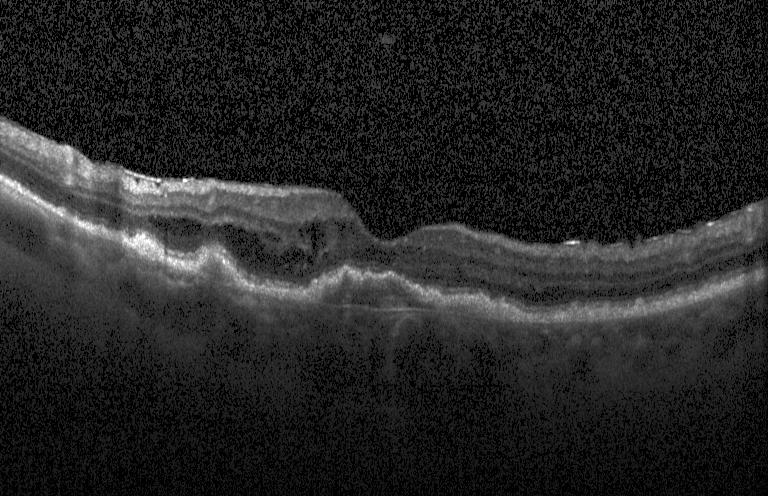
Optical coherence tomography scan
Macular OCT: a choroidal neovascular membrane.